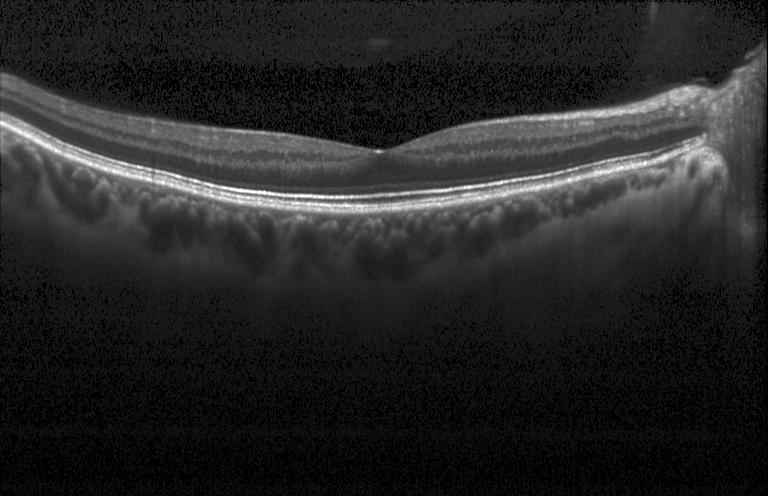

Macular OCT: no evidence of choroidal neovascularization, diabetic macular edema, or drusen.